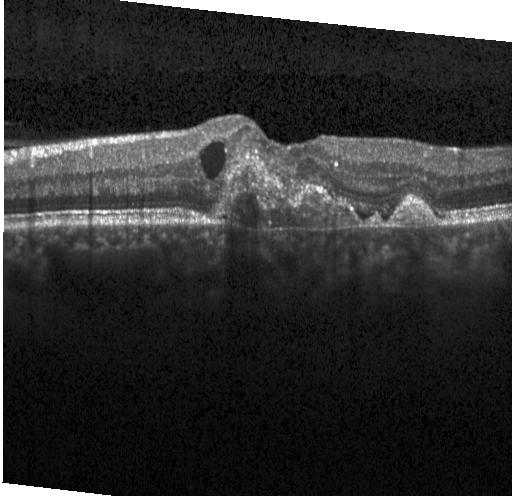
Retinal OCT cross-section
Dx: a choroidal neovascular membrane.